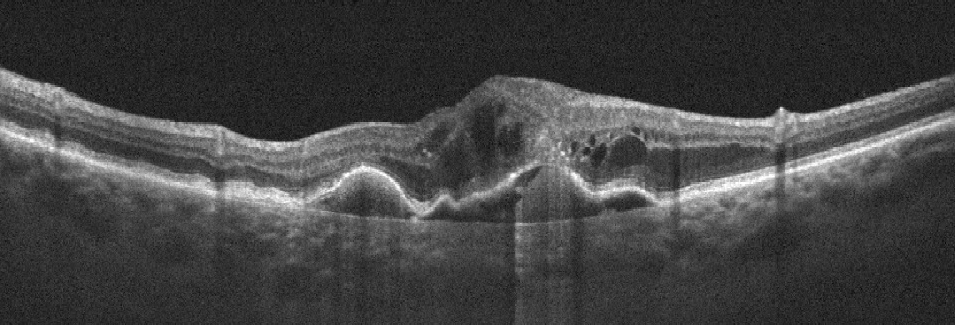

Optical coherence tomography scan. Finding: age-related macular degeneration (AMD).